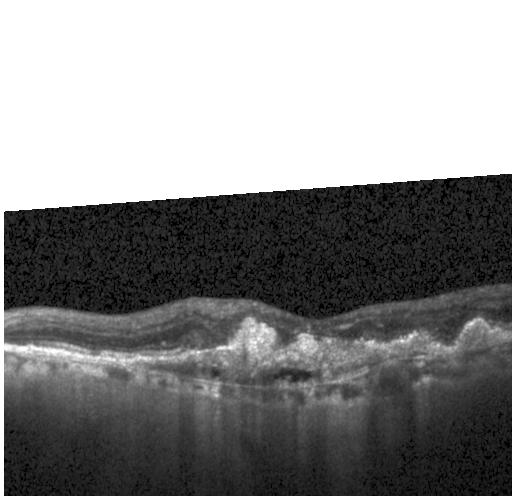 Optical coherence tomography B-scan
Impression: choroidal neovascularization.